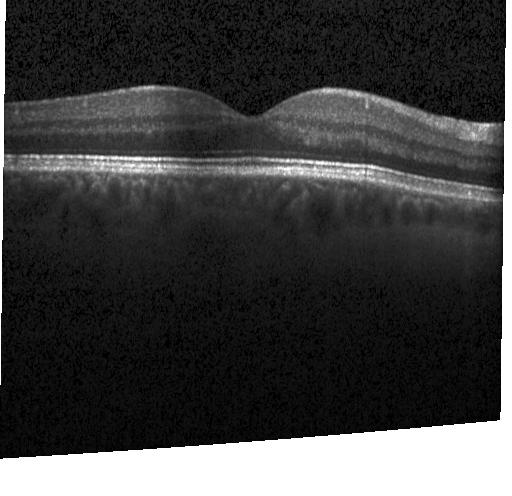

OCT B-scan.
Macular OCT: no evidence of choroidal neovascularization, diabetic macular edema, or drusen.